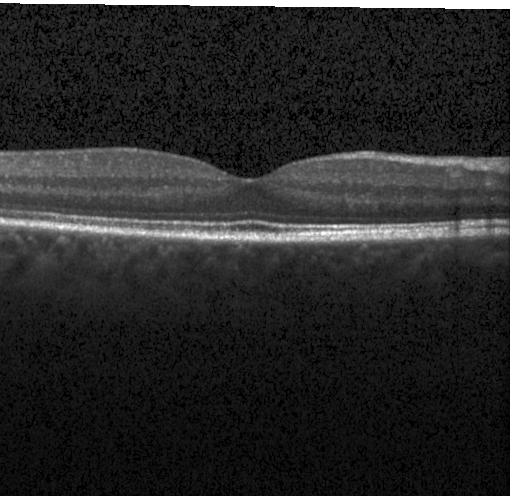 OCT B-scan, instrument: Heidelberg Spectralis, macular scan, spectral-domain optical coherence tomography
Impression: neither choroidal neovascularization, diabetic macular edema, nor drusen.